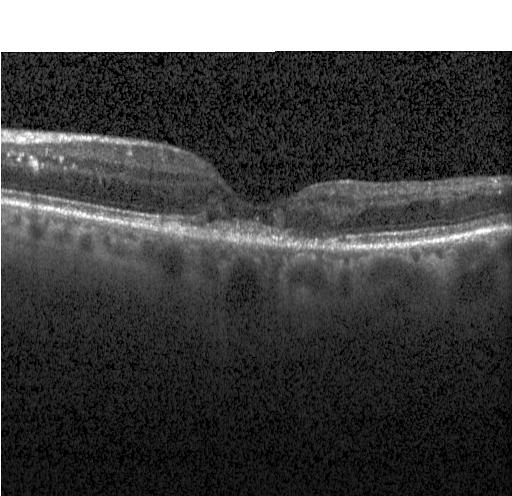
Macular scan. Heidelberg Spectralis. SD-OCT. Retinal OCT B-scan — Assessment: a choroidal neovascular membrane.